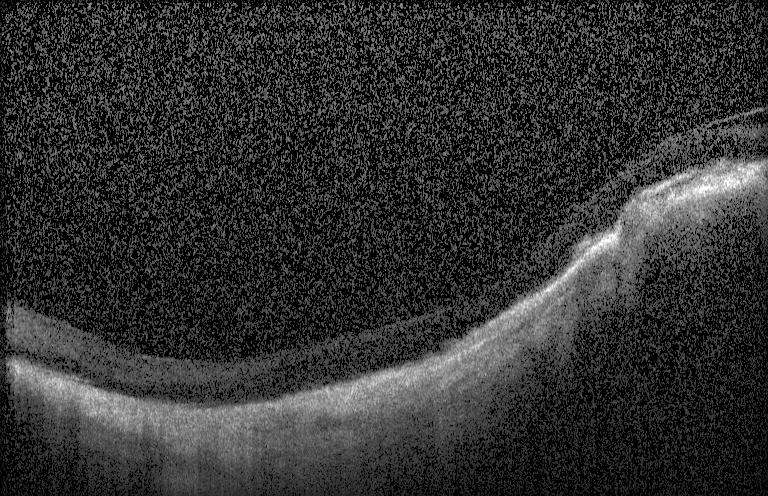 Optical coherence tomography scan. Heidelberg Spectralis OCT system. Macular scan.
Impression: choroidal neovascularization (CNV).